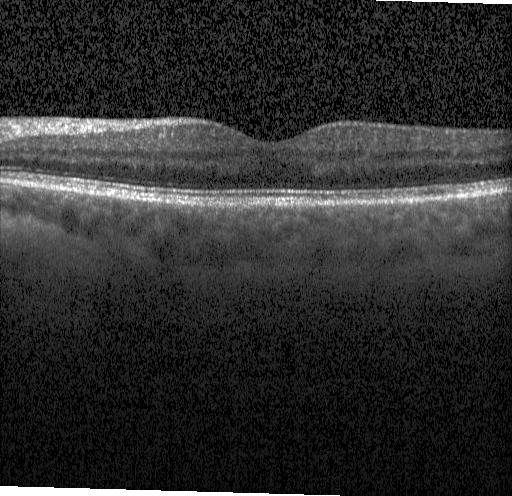

OCT line scan
Macular OCT: neither choroidal neovascularization, diabetic macular edema, nor drusen.